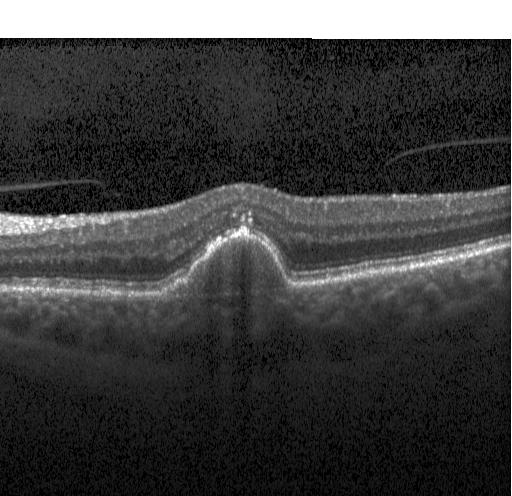

Heidelberg Spectralis OCT system; optical coherence tomography B-scan; through the macula
Diagnosis: CNV.